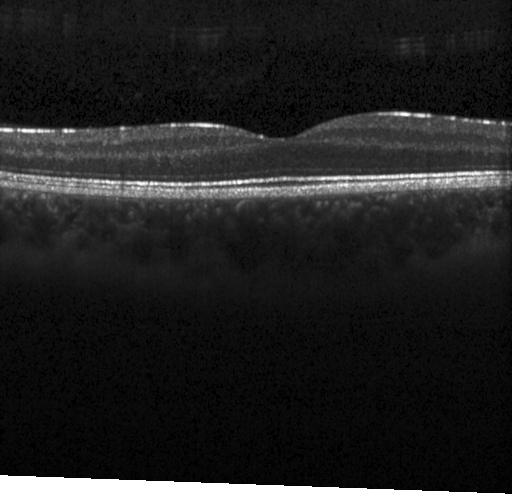

Retinal OCT cross-section · Heidelberg Spectralis OCT system · spectral-domain OCT · horizontal scan through the fovea — Macular OCT: neither choroidal neovascularization, diabetic macular edema, nor drusen.